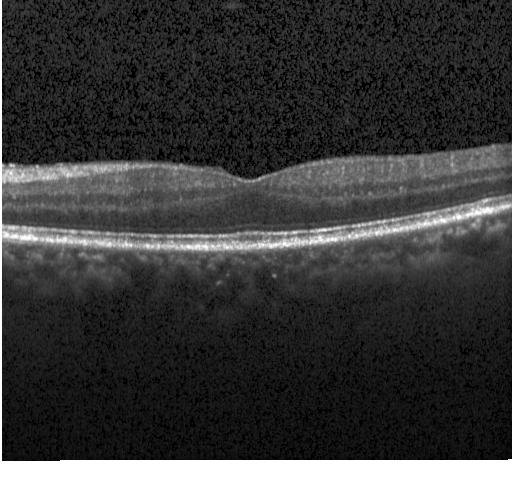 Optical coherence tomography B-scan; Heidelberg Spectralis; spectral-domain optical coherence tomography; centered on the fovea
This B-scan demonstrates no choroidal neovascularization, diabetic macular edema, or drusen.